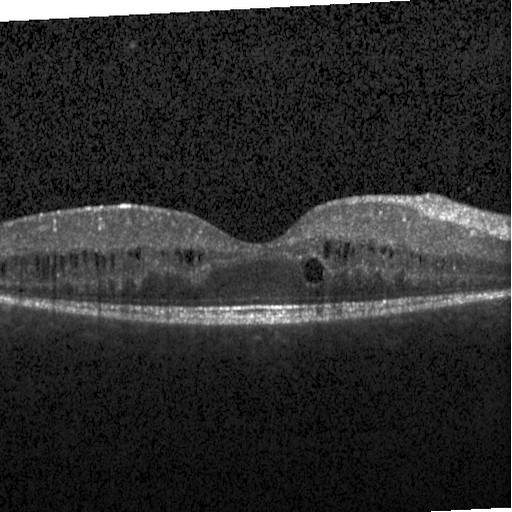 Retinal OCT B-scan
The scan shows diabetic macular edema (DME).